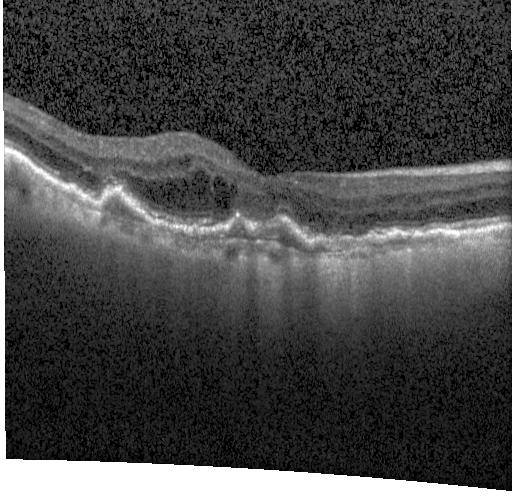
Retinal OCT cross-section — Diagnosis: choroidal neovascularization (CNV).